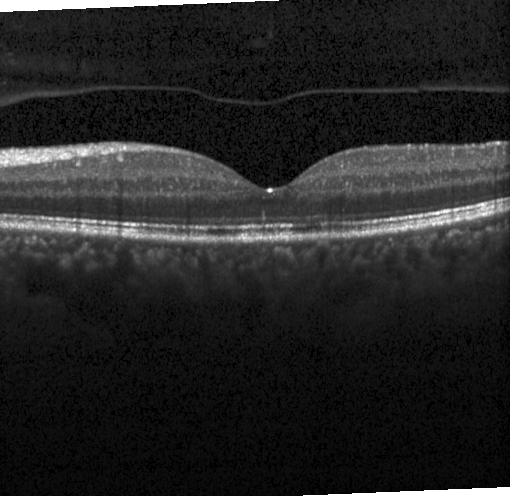

Impression: no evidence of choroidal neovascularization, diabetic macular edema, or drusen.